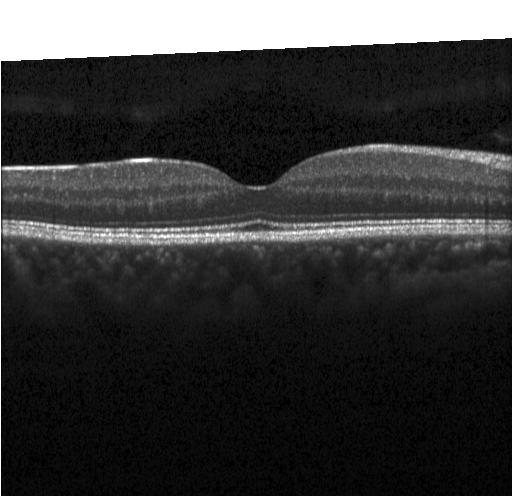 OCT line scan.
No evidence of choroidal neovascularization, diabetic macular edema, or drusen.